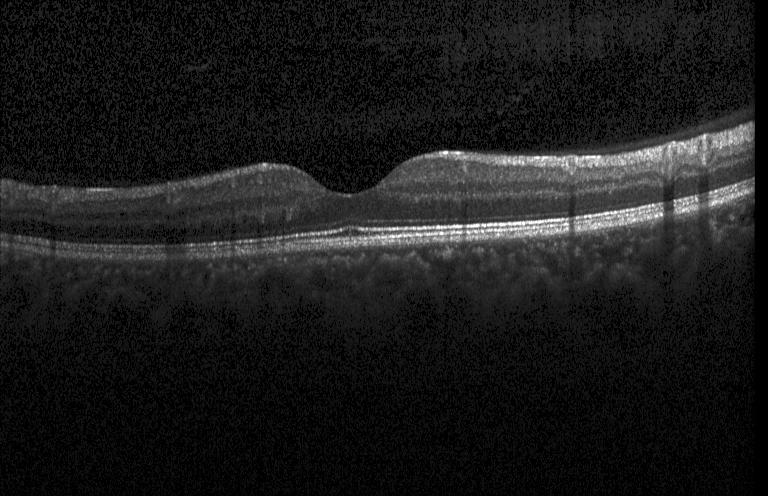 Assessment: no choroidal neovascularization, diabetic macular edema, or drusen.